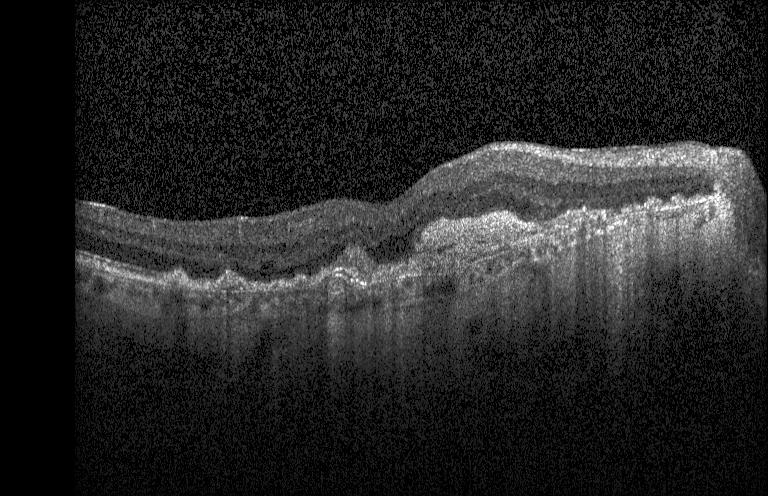

OCT B-scan showing choroidal neovascularization.